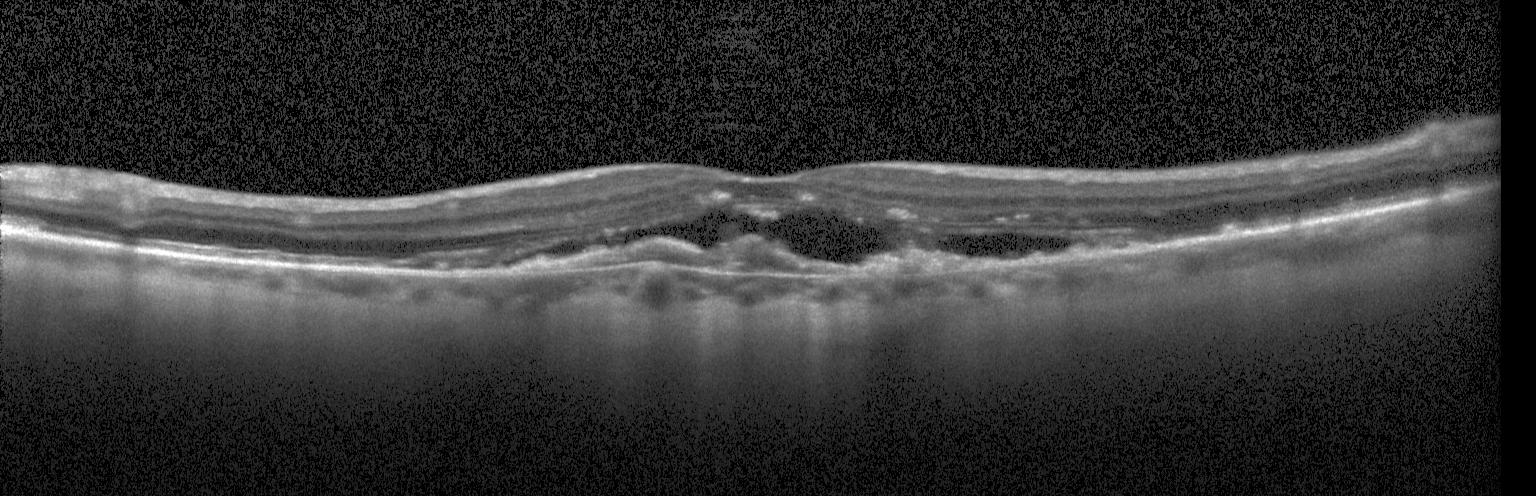
Heidelberg Spectralis OCT system; spectral-domain OCT; centered on the fovea; optical coherence tomography B-scan
Impression: choroidal neovascularization.